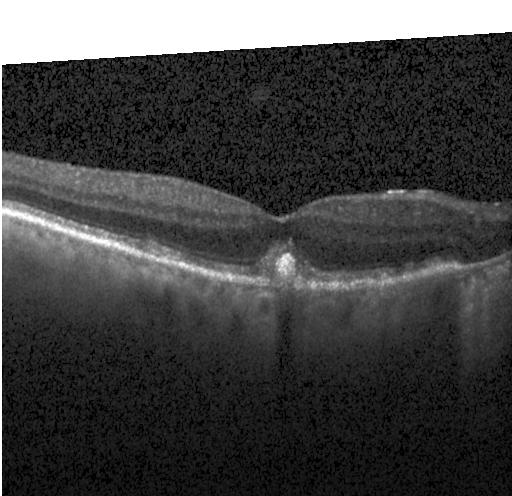
Spectral-domain OCT, Heidelberg Spectralis OCT system, horizontal scan through the fovea, optical coherence tomography scan. Macular OCT: choroidal neovascularization (CNV).